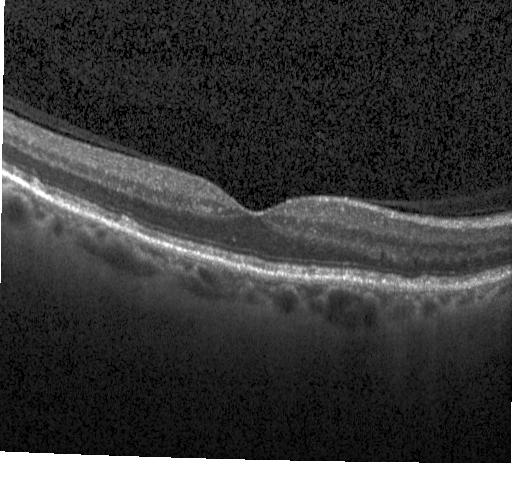

Optical coherence tomography B-scan — Assessment: no choroidal neovascularization, no diabetic macular edema, and no drusen.